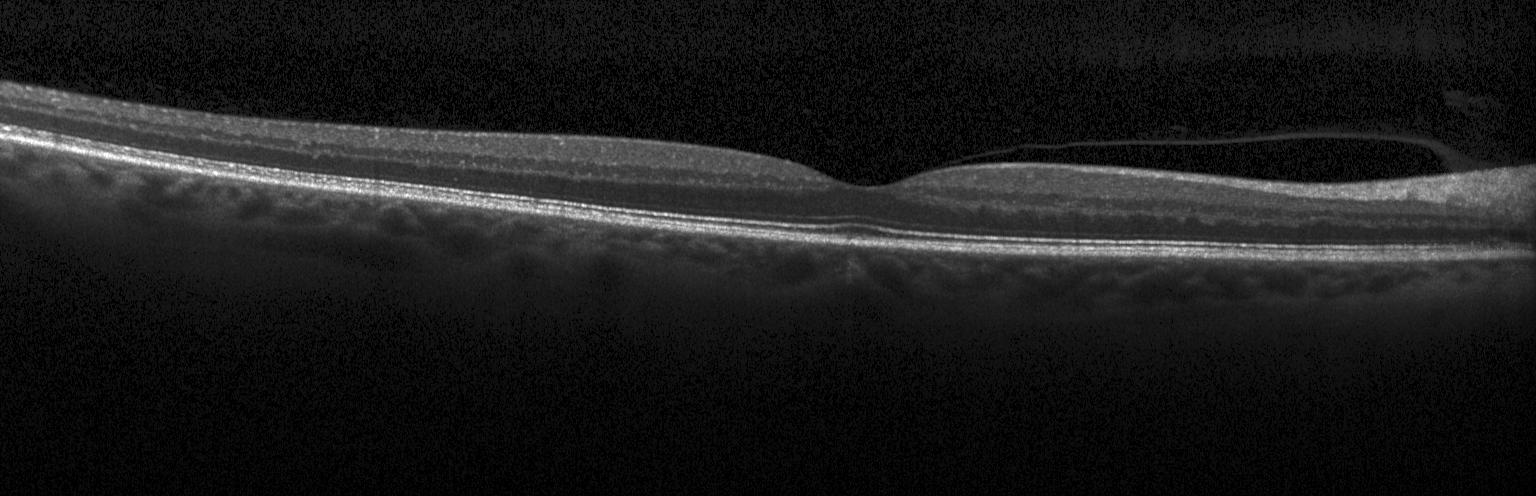
Heidelberg Spectralis OCT system, OCT line scan, centered on the fovea. Finding: no choroidal neovascularization, diabetic macular edema, or drusen.